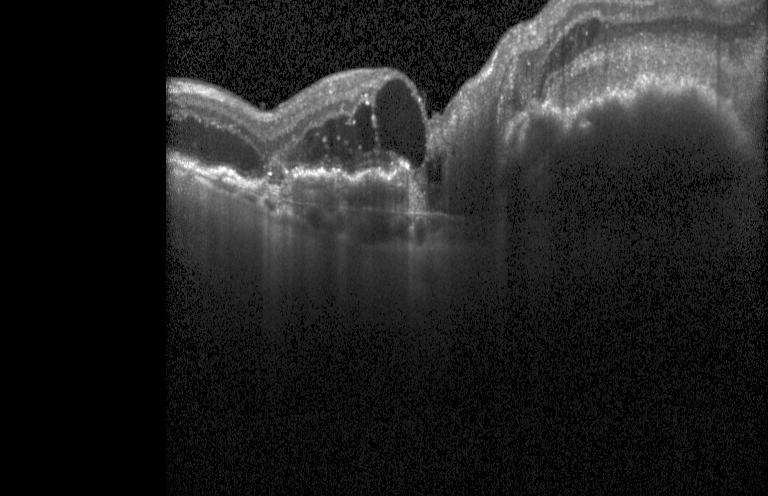 OCT B-scan
The scan shows CNV.